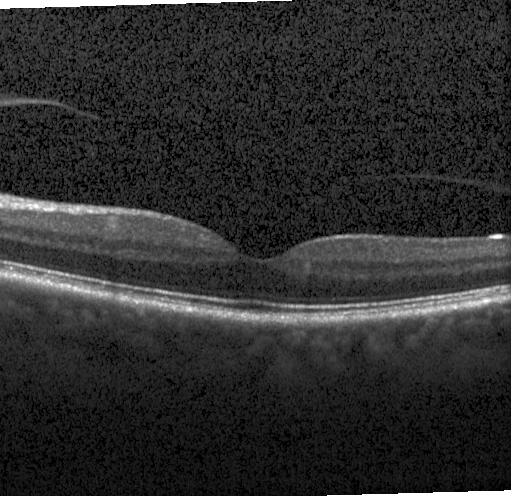
Dx: no evidence of choroidal neovascularization, diabetic macular edema, or drusen.